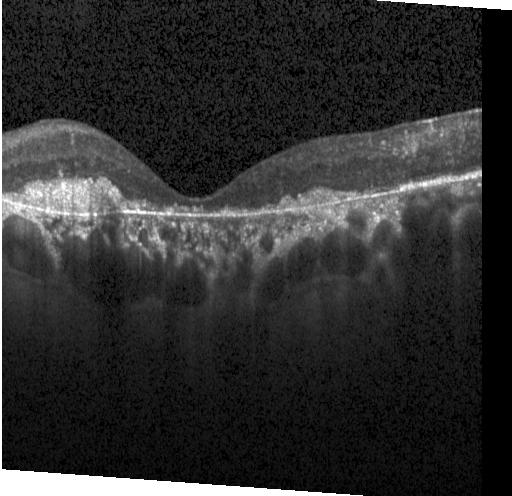

Instrument: Heidelberg Spectralis; spectral-domain optical coherence tomography; centered on the fovea; retinal OCT cross-section — The scan shows a choroidal neovascular membrane.